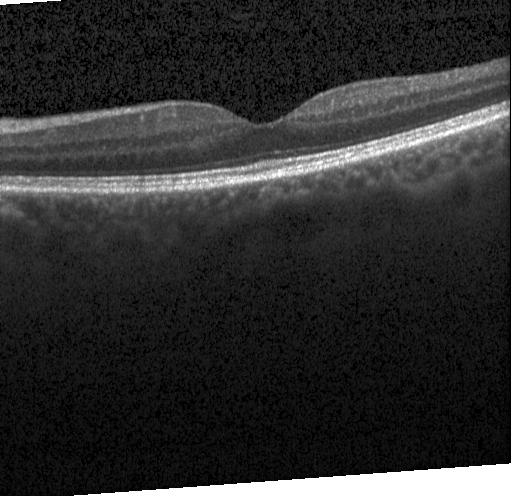 Retinal OCT cross-section showing neither choroidal neovascularization, diabetic macular edema, nor drusen.